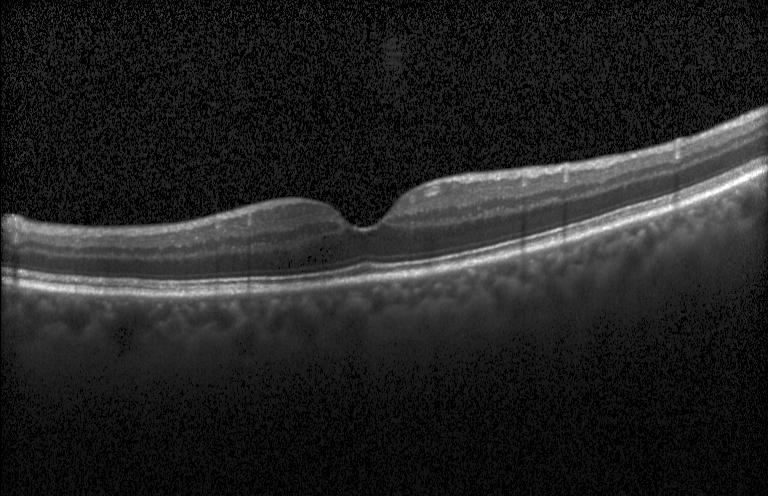

Finding: no choroidal neovascularization, diabetic macular edema, or drusen.